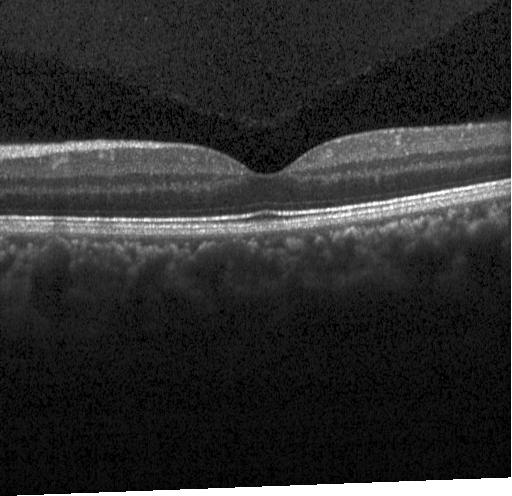 This B-scan demonstrates neither choroidal neovascularization, diabetic macular edema, nor drusen.